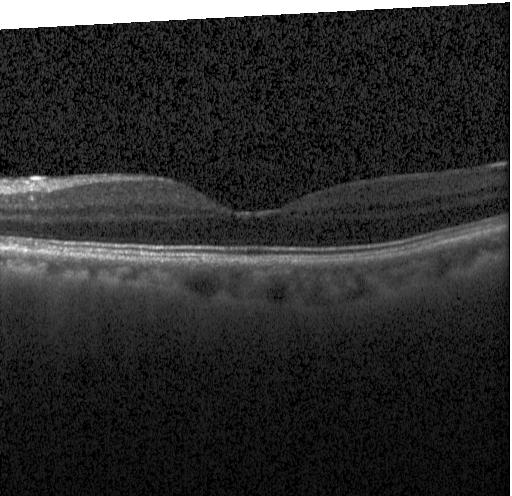

SD-OCT. Optical coherence tomography scan. Centered on the fovea
Finding: no choroidal neovascularization, diabetic macular edema, or drusen.